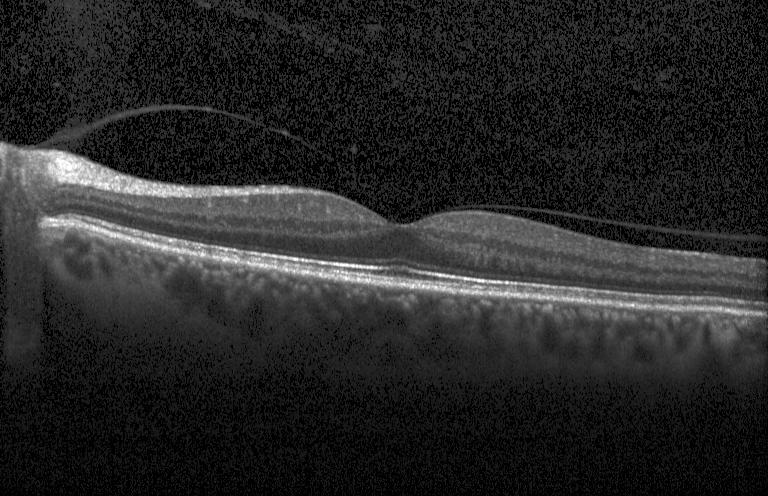

Macular scan, optical coherence tomography B-scan.
This B-scan demonstrates no evidence of choroidal neovascularization, diabetic macular edema, or drusen.